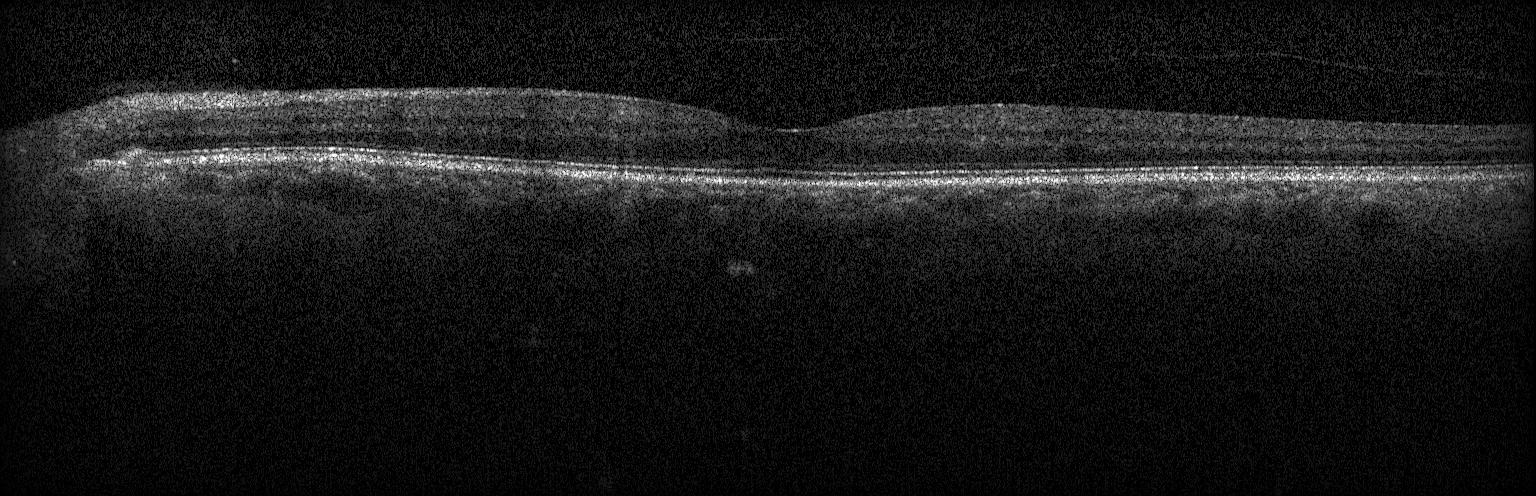
SD-OCT; optical coherence tomography B-scan; instrument: Heidelberg Spectralis
The scan shows neither choroidal neovascularization, diabetic macular edema, nor drusen.